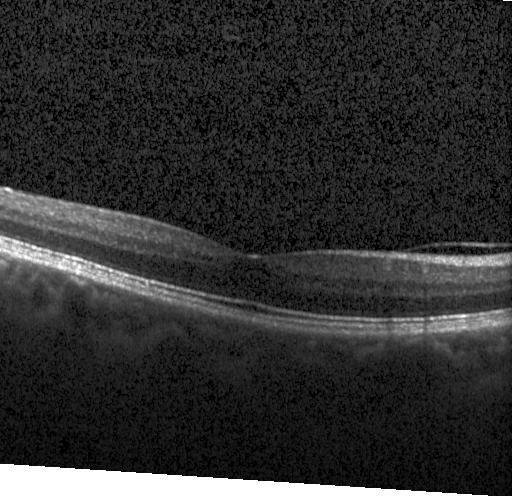 Diagnosis: neither choroidal neovascularization, diabetic macular edema, nor drusen.